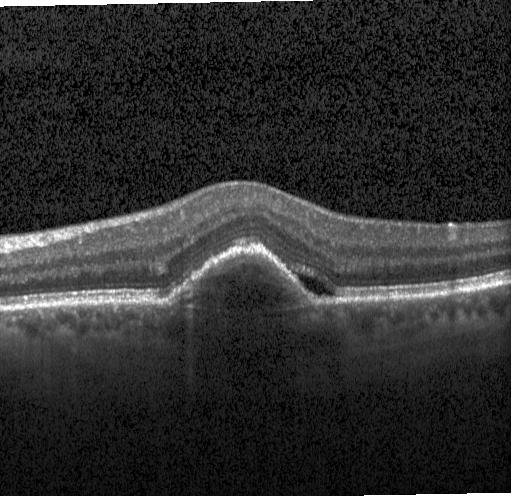
Impression: a choroidal neovascular membrane.